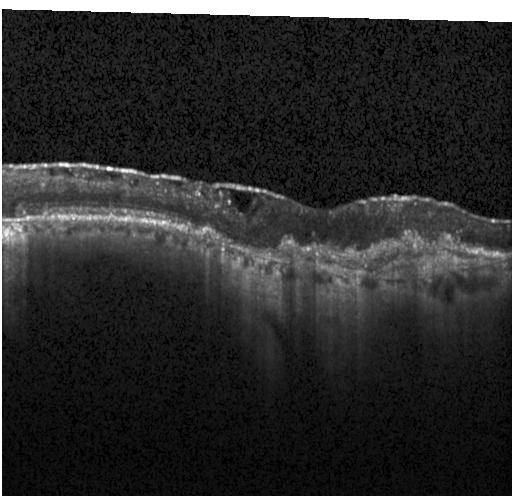
OCT scan showing a choroidal neovascular membrane.